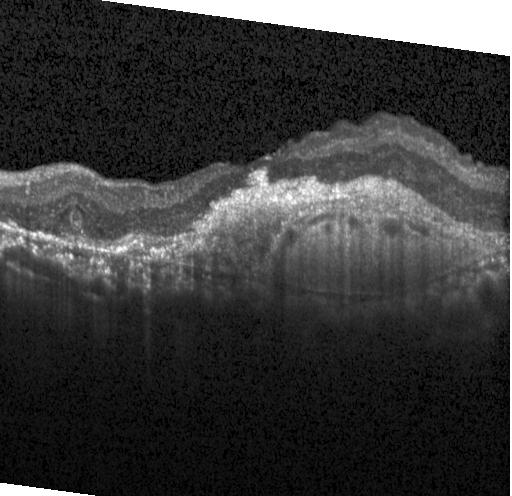 This B-scan demonstrates choroidal neovascularization.